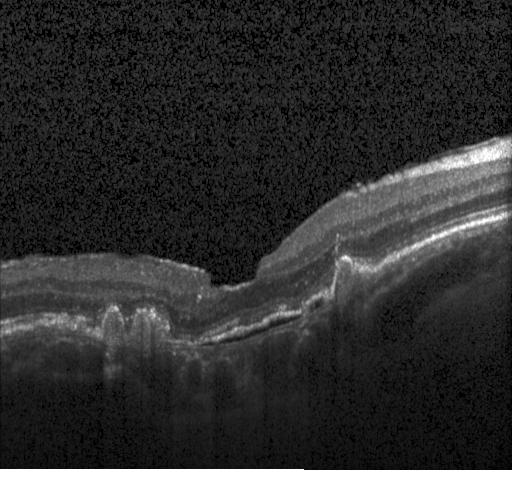 Finding: a choroidal neovascular membrane.